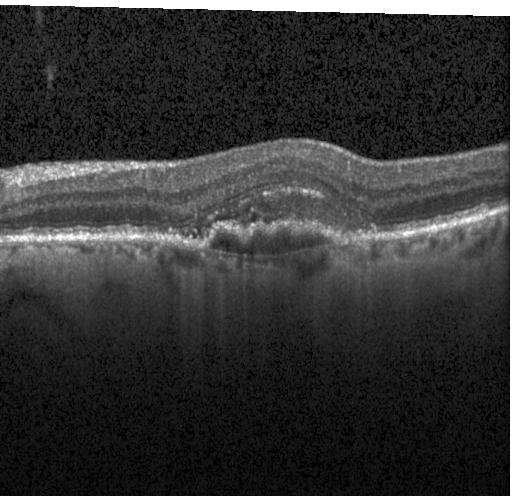
Retinal OCT B-scan, through the macula — OCT finding: choroidal neovascularization.